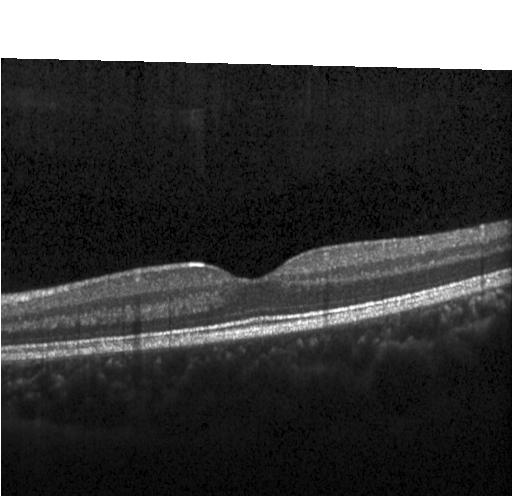

Centered on the fovea · optical coherence tomography scan.
Assessment: no choroidal neovascularization, no diabetic macular edema, and no drusen.